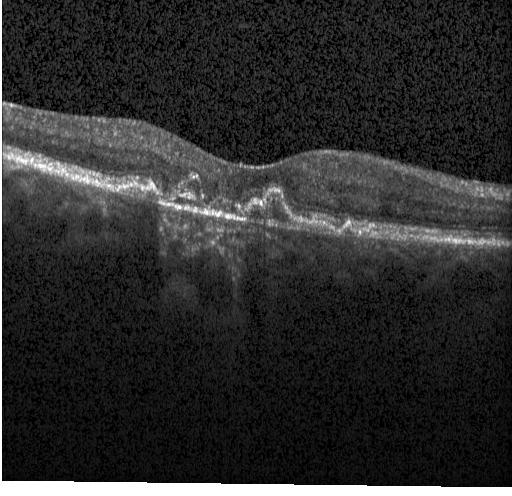

Finding: choroidal neovascularization.